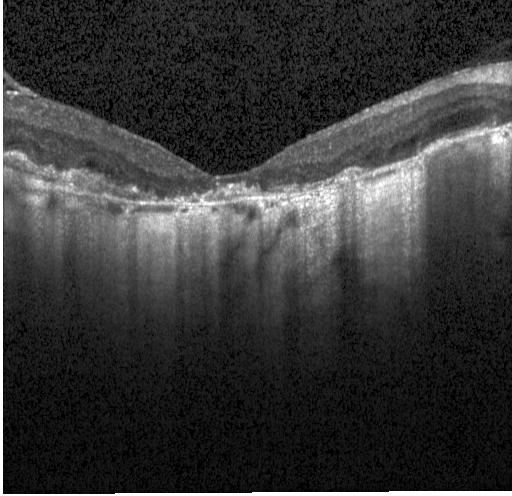
Spectral-domain optical coherence tomography, retinal OCT cross-section.
Diagnosis: choroidal neovascularization (CNV).